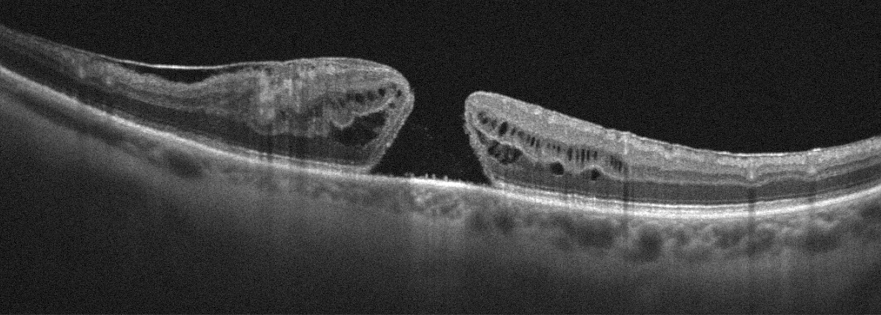
Through the macula, OCT B-scan — The scan shows VID.